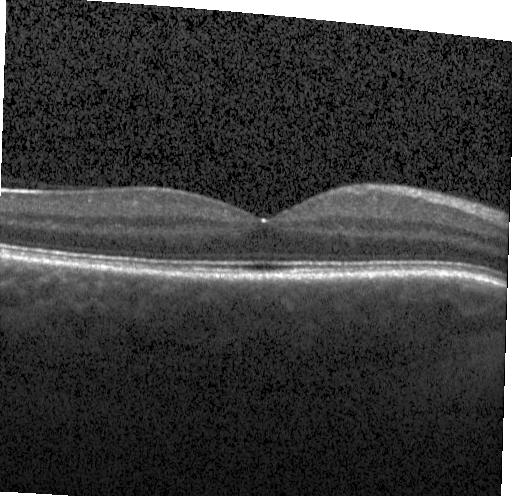

SD-OCT. Instrument: Heidelberg Spectralis. Retinal OCT cross-section.
No choroidal neovascularization, no diabetic macular edema, and no drusen.